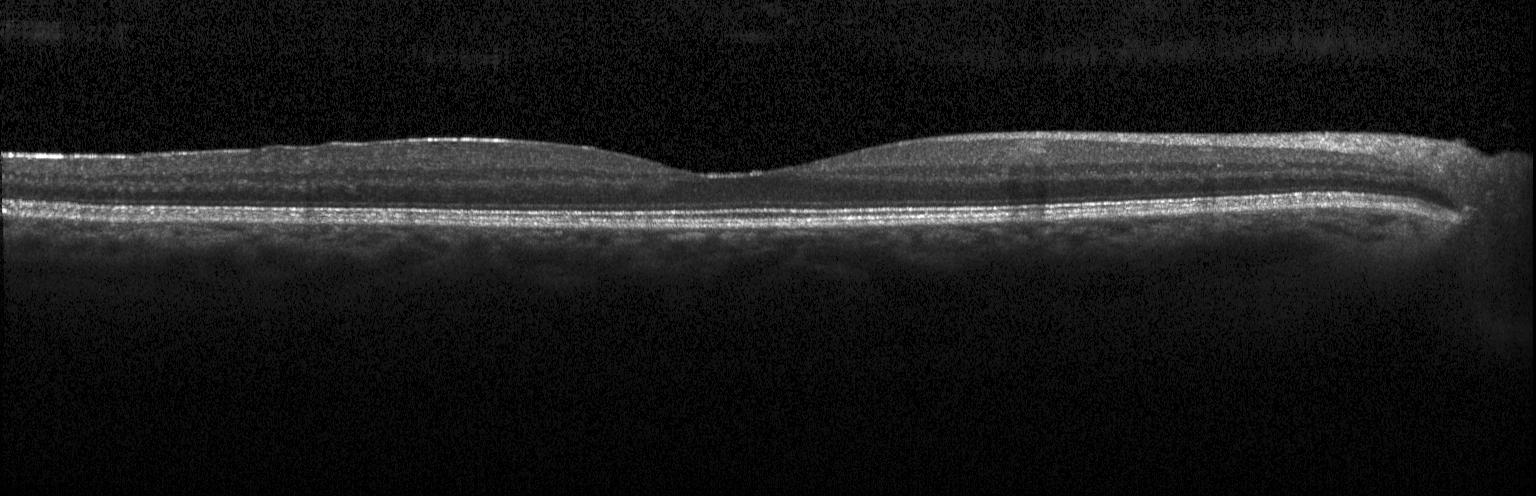 Instrument: Heidelberg Spectralis; spectral-domain OCT; horizontal scan through the fovea; optical coherence tomography B-scan.
Impression: no evidence of choroidal neovascularization, diabetic macular edema, or drusen.